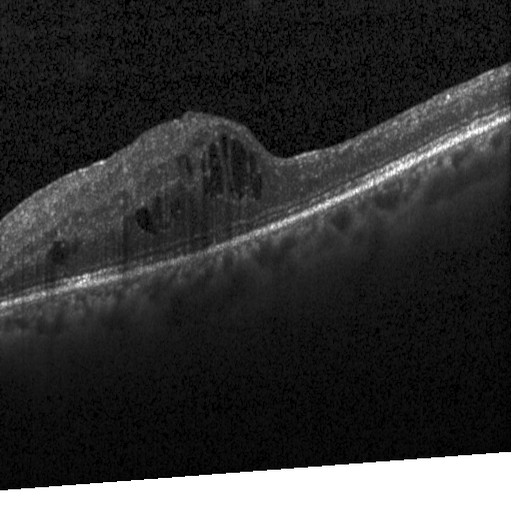

Spectral-domain OCT; retinal OCT B-scan
The scan shows diabetic macular edema (DME).